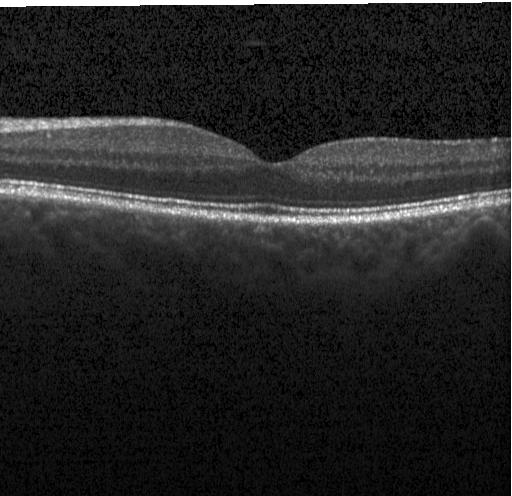 Fovea-centered. OCT B-scan
Impression: no evidence of choroidal neovascularization, diabetic macular edema, or drusen.